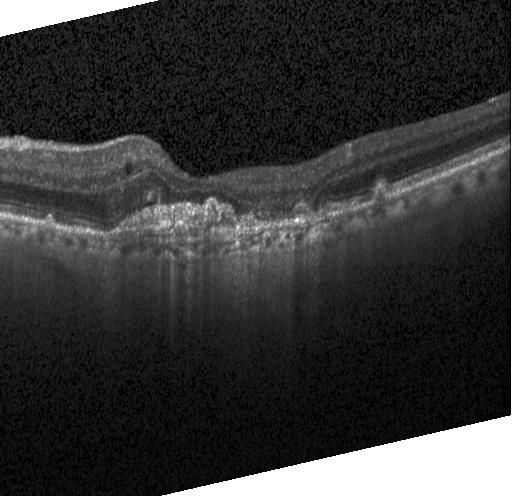

Finding: CNV.